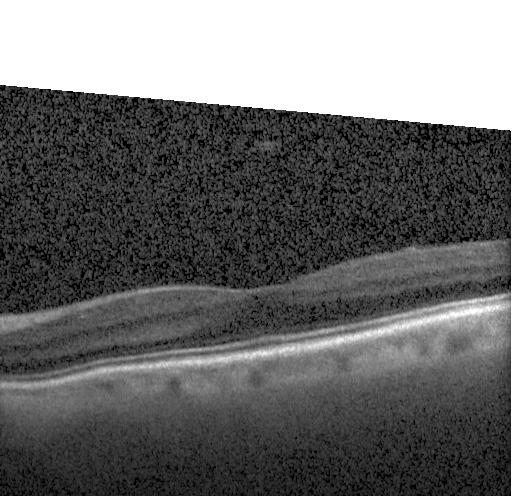
OCT scan showing no CNV, DME, or drusen.